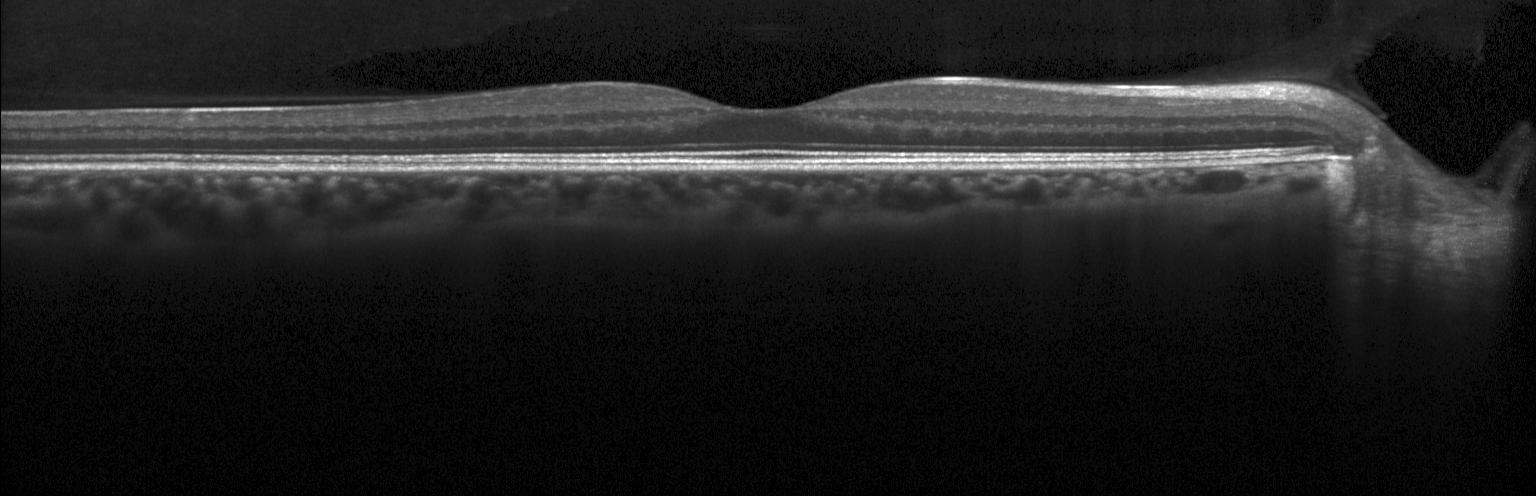

Centered on the fovea · OCT line scan · Heidelberg Spectralis · spectral-domain optical coherence tomography.
OCT finding: neither CNV, DME, nor drusen.